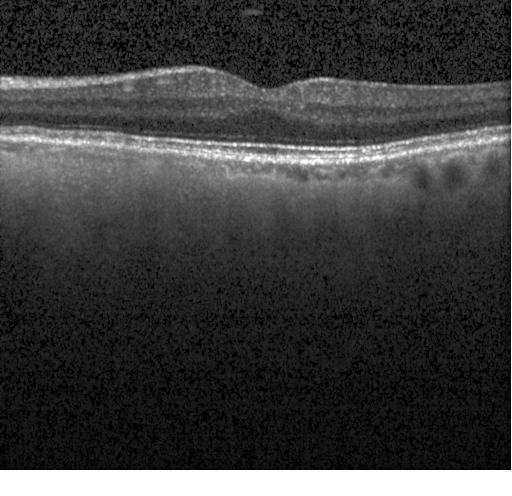

Fovea-centered · SD-OCT · OCT B-scan · instrument: Heidelberg Spectralis — Diagnosis: no choroidal neovascularization, no diabetic macular edema, and no drusen.